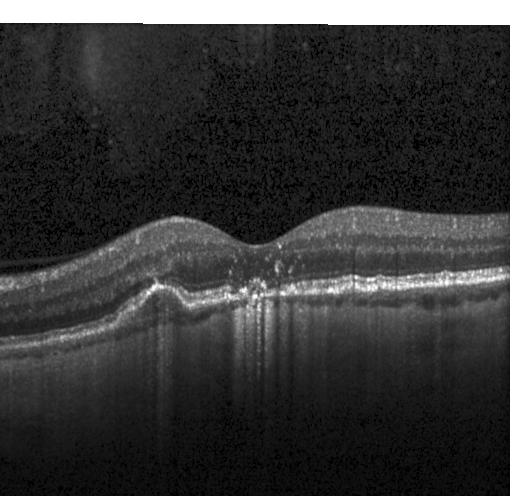 Diagnosis: a choroidal neovascular membrane.